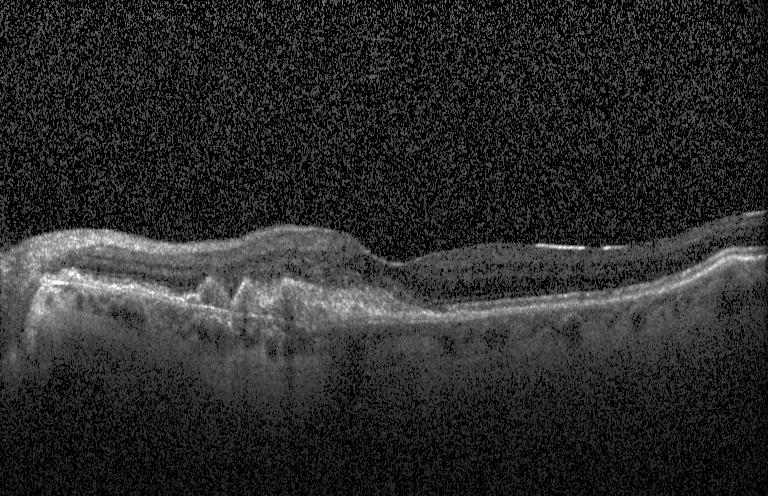

Optical coherence tomography scan. Fovea-centered. Spectral-domain OCT. Finding: CNV.